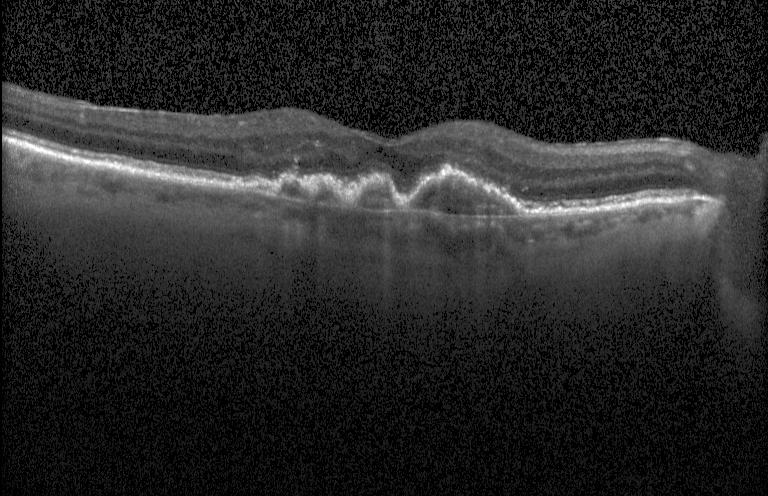

Assessment: choroidal neovascularization (CNV).